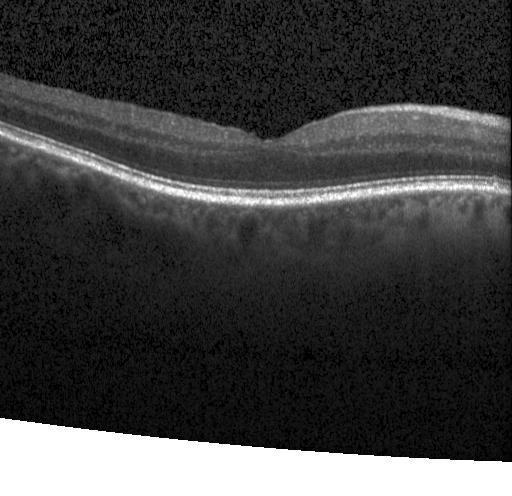
Finding: no choroidal neovascularization, no diabetic macular edema, and no drusen.